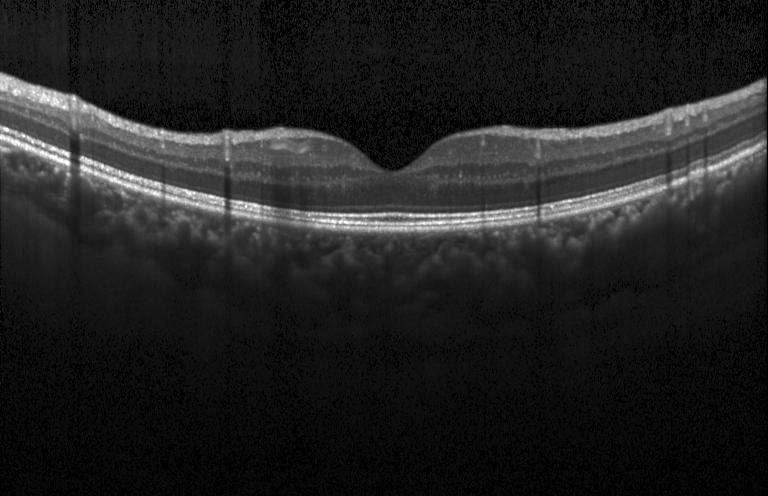

OCT finding: neither choroidal neovascularization, diabetic macular edema, nor drusen.